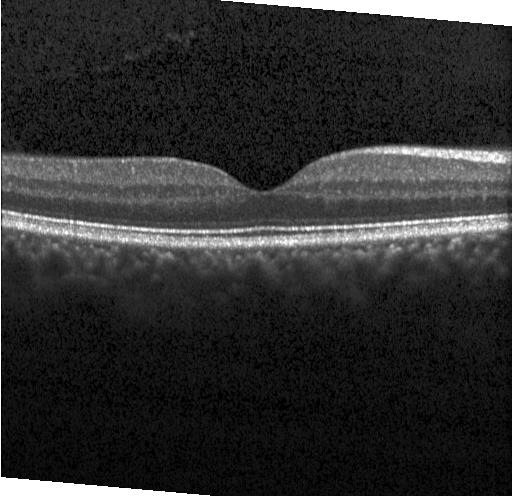 Acquired on a Heidelberg Spectralis · retinal OCT B-scan. No evidence of CNV, DME, or drusen.